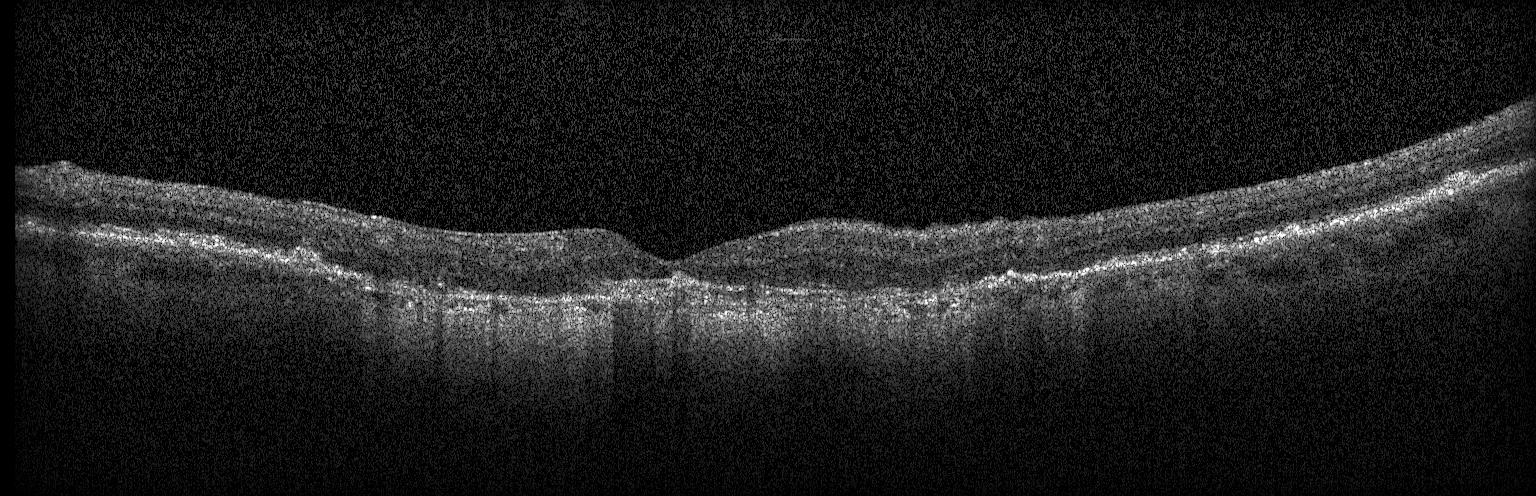 Spectral-domain optical coherence tomography, OCT line scan, through the macula — The scan shows a choroidal neovascular membrane.